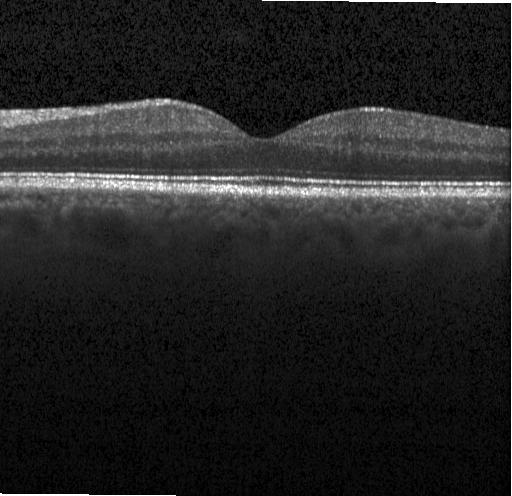 OCT line scan; SD-OCT; acquired on a Heidelberg Spectralis.
The scan shows no choroidal neovascularization, diabetic macular edema, or drusen.